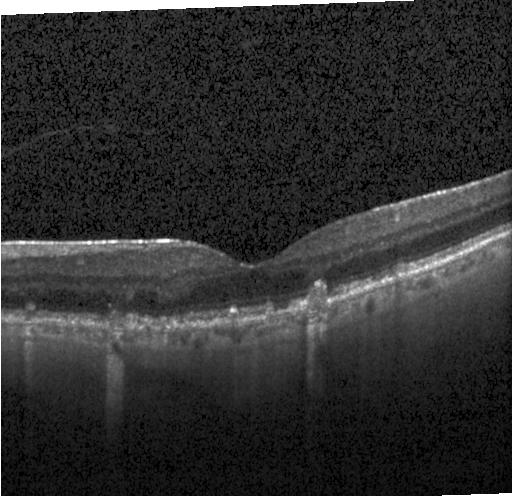 Assessment: drusen.